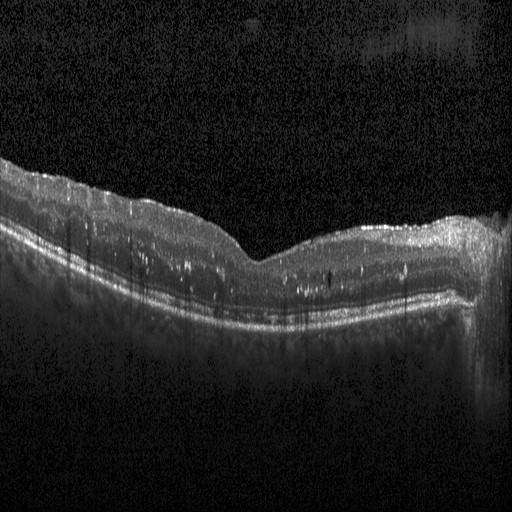

Retinal OCT B-scan. Diagnosis: diabetic macular edema (DME).